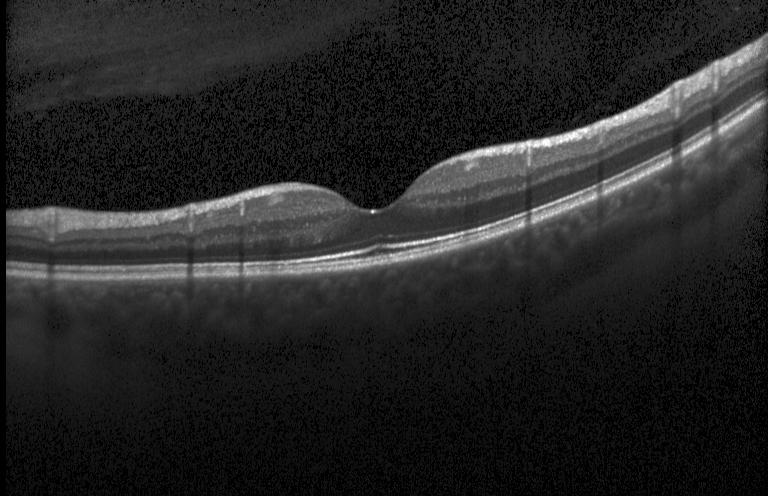
Dx: no choroidal neovascularization, no diabetic macular edema, and no drusen.